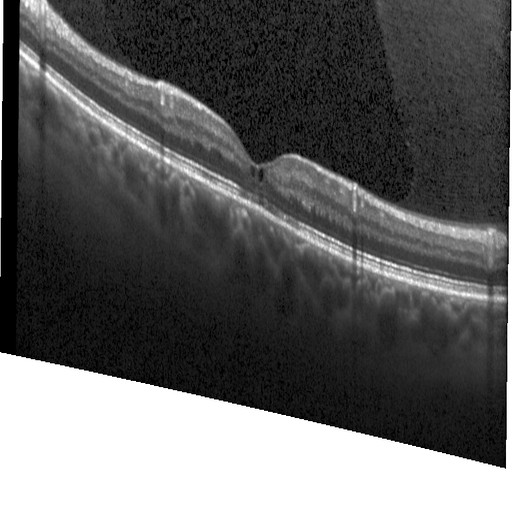

The scan shows diabetic macular edema.